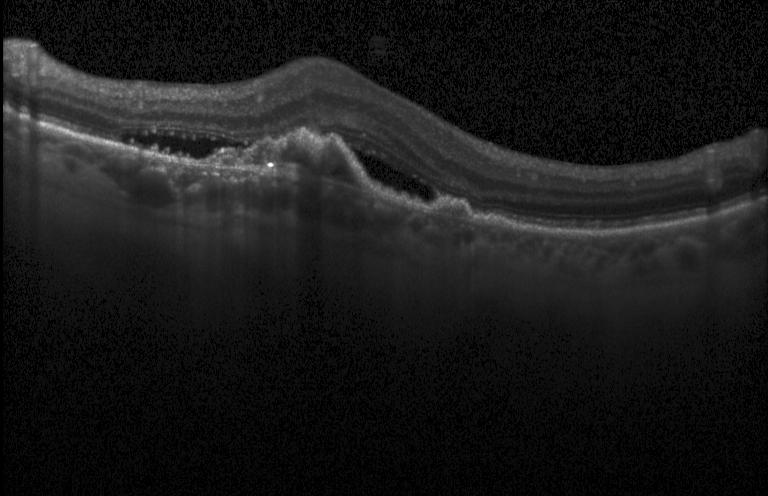
This B-scan demonstrates CNV.